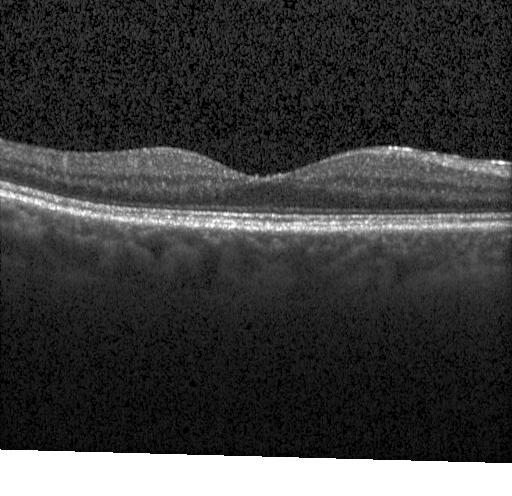

OCT B-scan
Dx: no choroidal neovascularization, diabetic macular edema, or drusen.